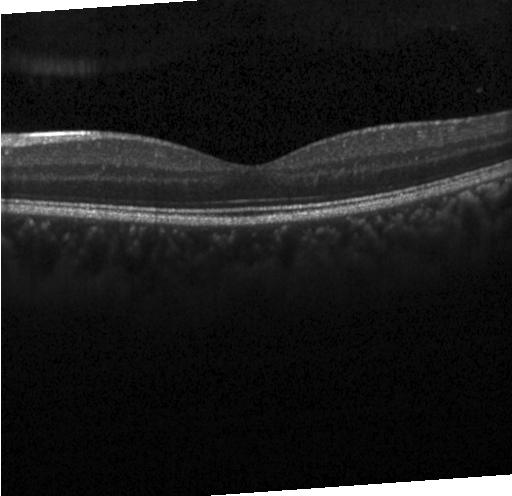

OCT line scan · macular scan — Finding: no evidence of choroidal neovascularization, diabetic macular edema, or drusen.